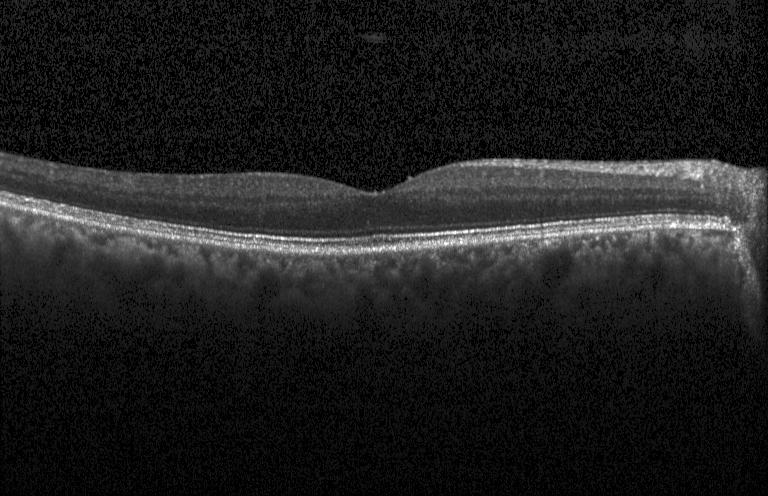

Centered on the fovea; acquired on a Heidelberg Spectralis; spectral-domain OCT; optical coherence tomography B-scan. No CNV, DME, or drusen.